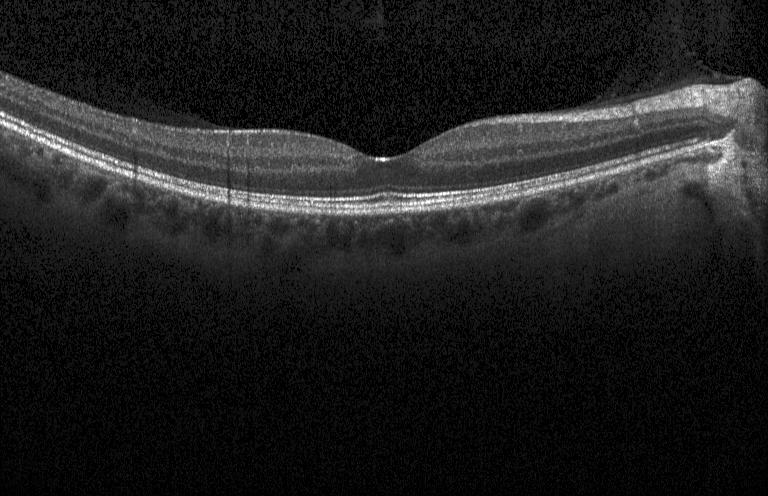
Optical coherence tomography B-scan — Impression: no evidence of choroidal neovascularization, diabetic macular edema, or drusen.